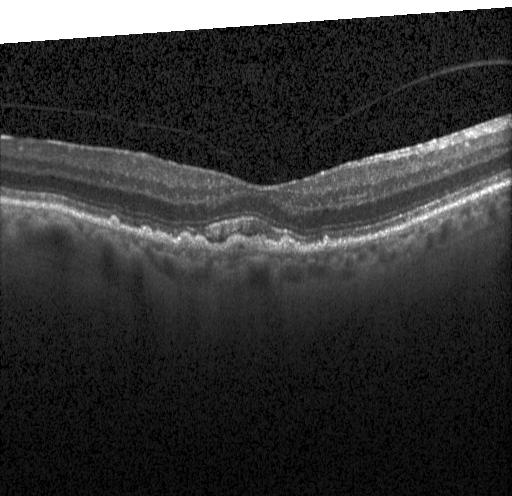
Dx: CNV.